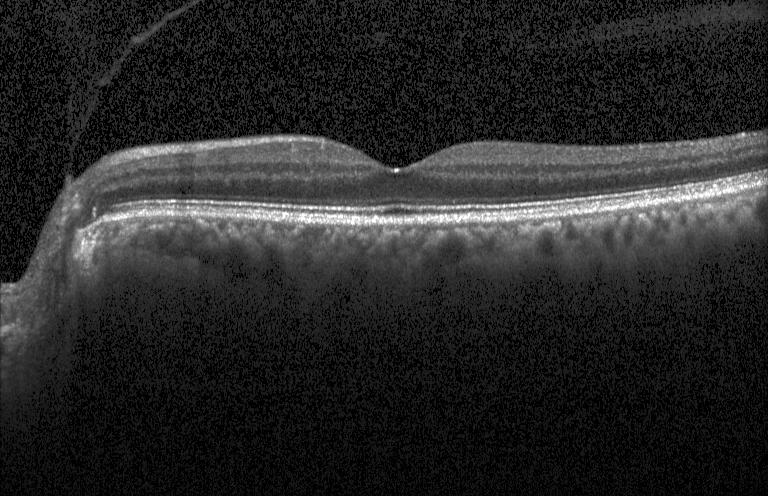 Optical coherence tomography scan · macular scan.
Finding: neither CNV, DME, nor drusen.